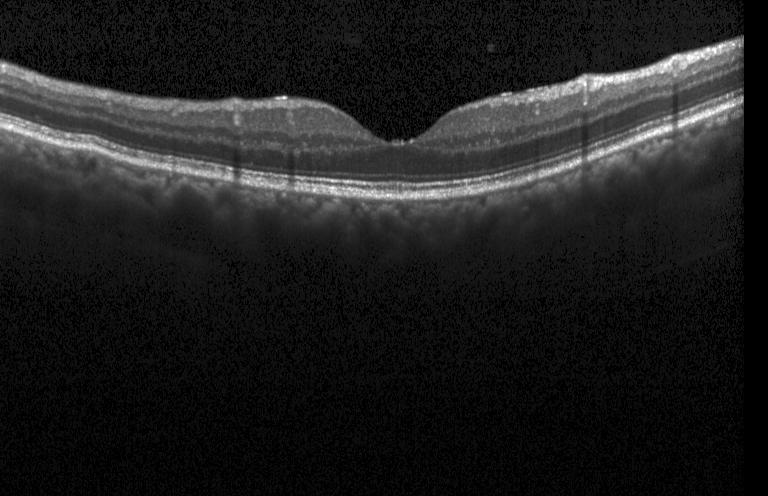 Horizontal scan through the fovea, optical coherence tomography scan, acquired on a Heidelberg Spectralis, spectral-domain OCT — Diagnosis: no choroidal neovascularization, diabetic macular edema, or drusen.